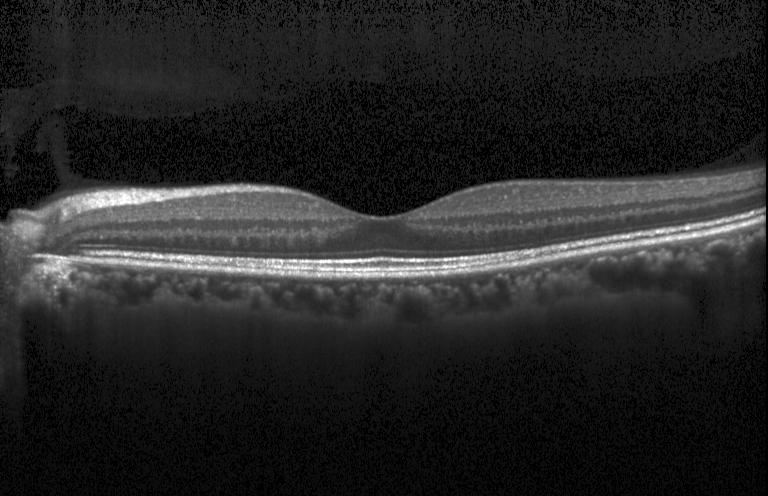

Fovea-centered · Heidelberg Spectralis · spectral-domain optical coherence tomography · retinal OCT cross-section.
The scan shows neither choroidal neovascularization, diabetic macular edema, nor drusen.